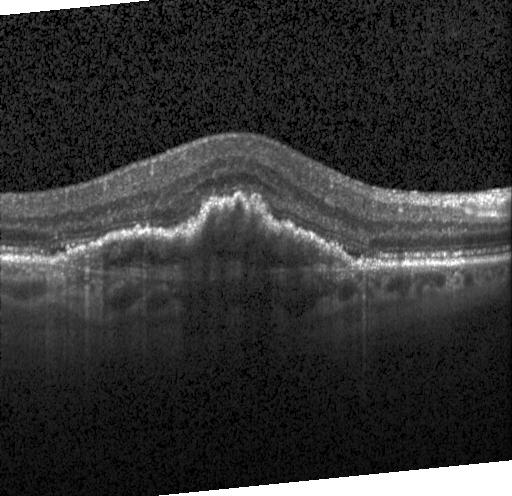 Retinal OCT cross-section; through the macula
Diagnosis: a choroidal neovascular membrane.